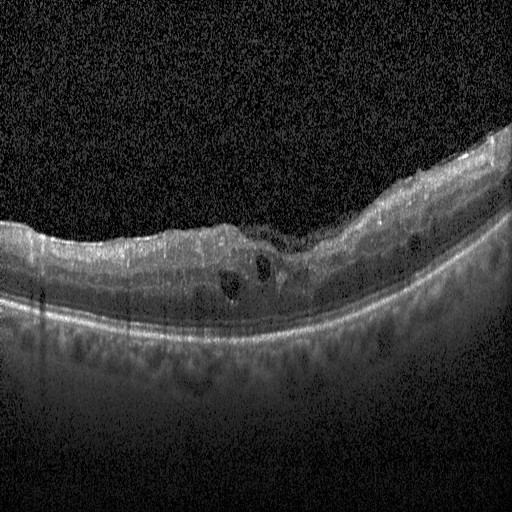 Spectral-domain optical coherence tomography. Instrument: Heidelberg Spectralis. Centered on the fovea. Retinal OCT cross-section. Dx: diabetic macular edema (DME).